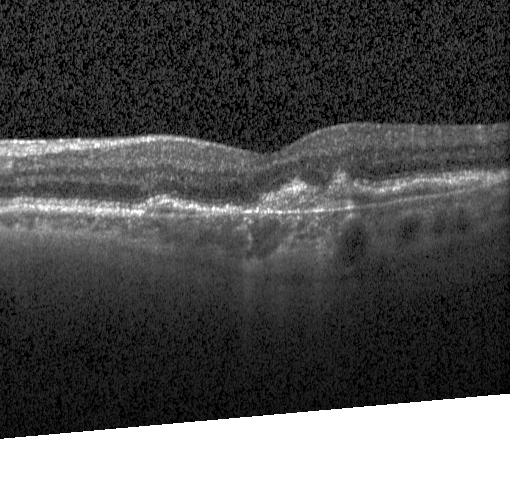

Optical coherence tomography B-scan · Heidelberg Spectralis OCT system · spectral-domain OCT — Impression: choroidal neovascularization (CNV).